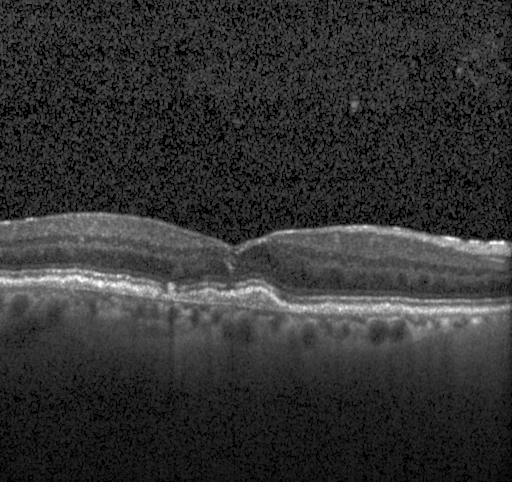 OCT scan showing a choroidal neovascular membrane.